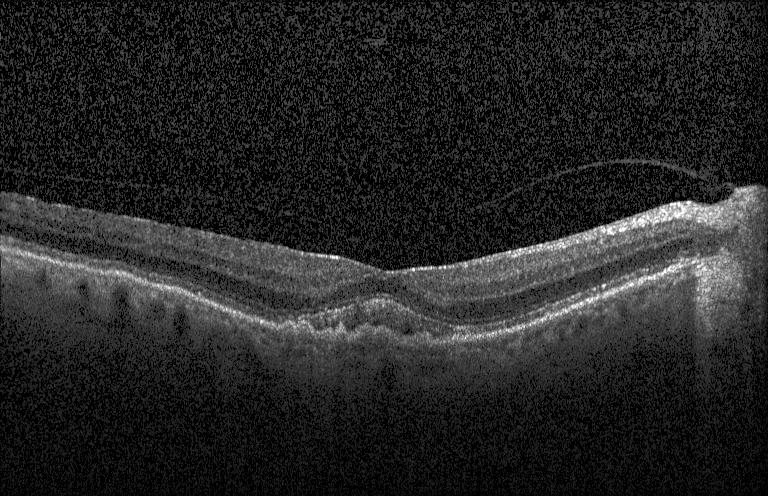

Retinal OCT cross-section; instrument: Heidelberg Spectralis.
Macular OCT: choroidal neovascularization.